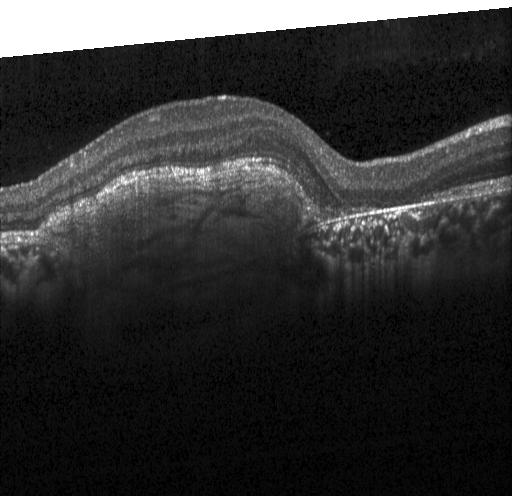
OCT line scan. A choroidal neovascular membrane.